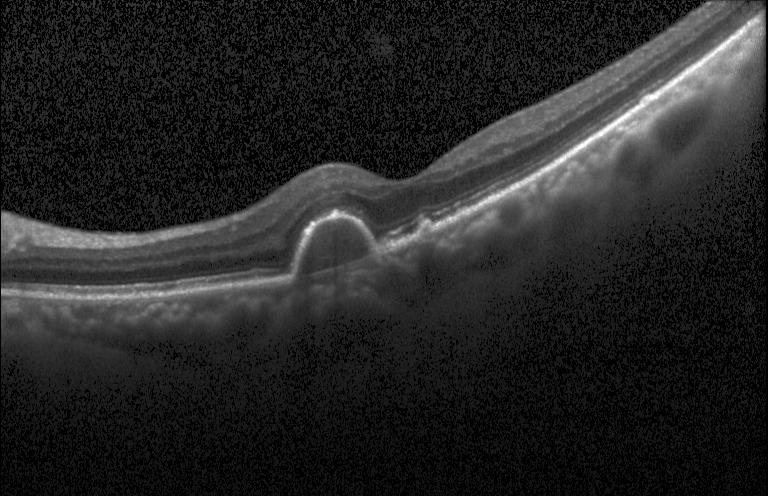 Diagnosis: multiple drusen.